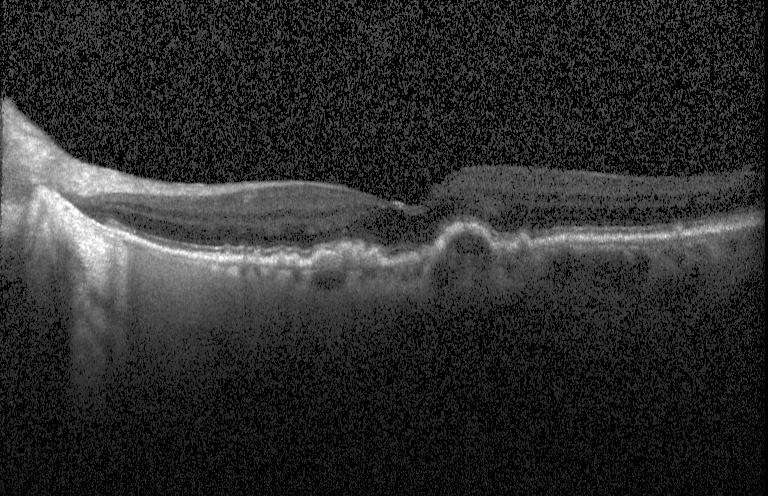
Spectral-domain OCT B-scan: CNV.